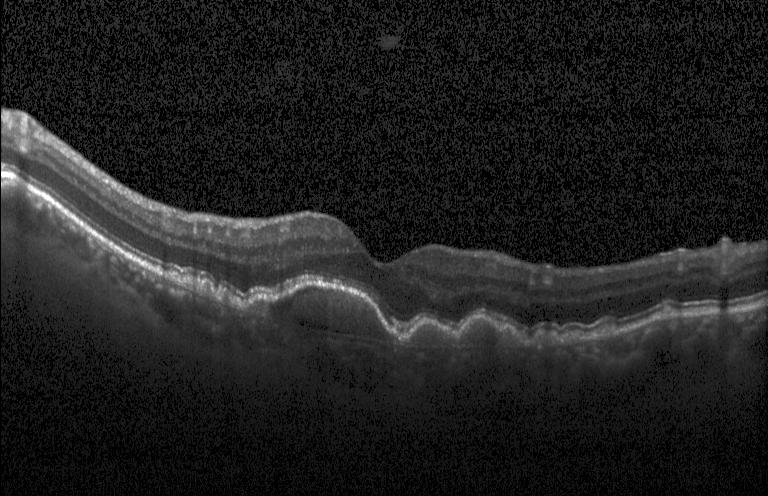
Retinal OCT B-scan, acquired on a Heidelberg Spectralis.
Macular OCT: drusen.